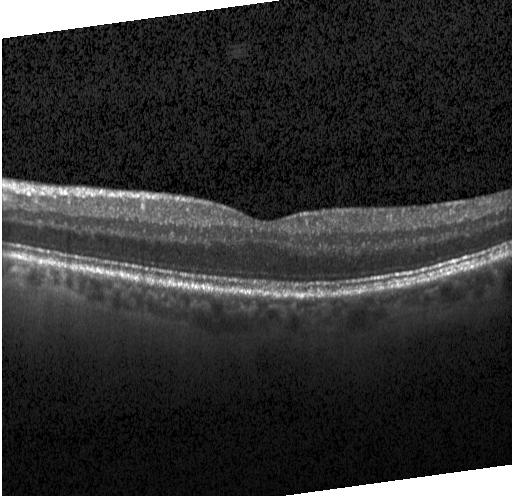
Dx: no choroidal neovascularization, diabetic macular edema, or drusen.